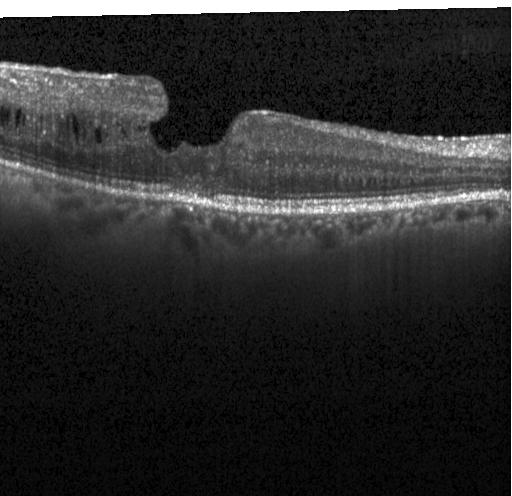 Spectral-domain optical coherence tomography; OCT line scan; macular scan
Dx: DME.